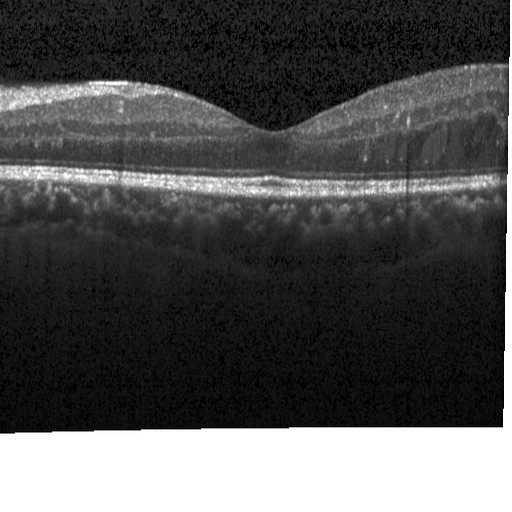

Dx: DME.